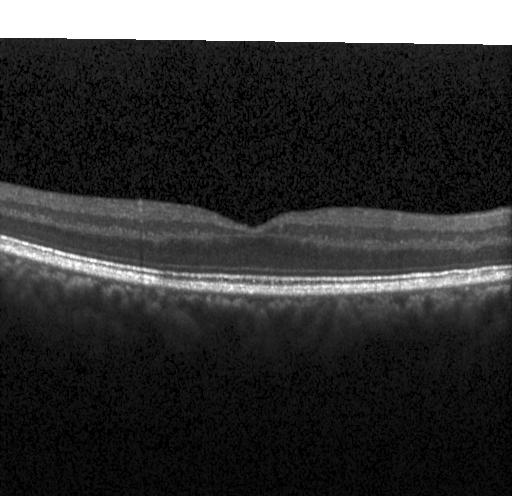
Spectral-domain optical coherence tomography, centered on the fovea, retinal OCT cross-section — The scan shows no CNV, DME, or drusen.